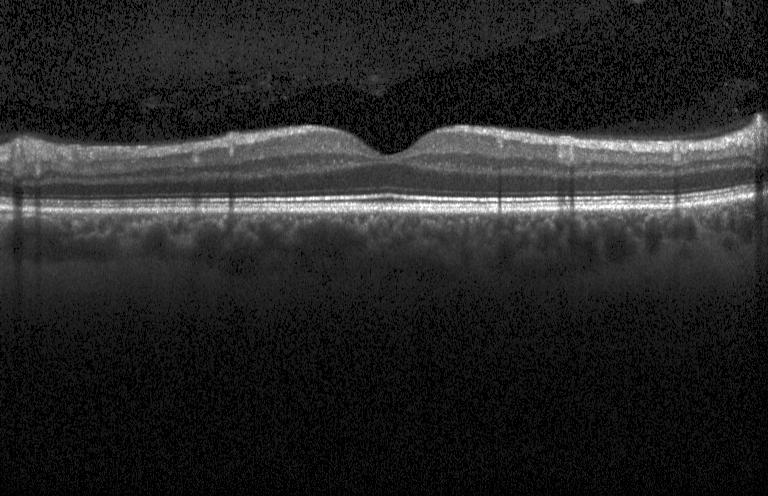
OCT finding: no choroidal neovascularization, no diabetic macular edema, and no drusen.